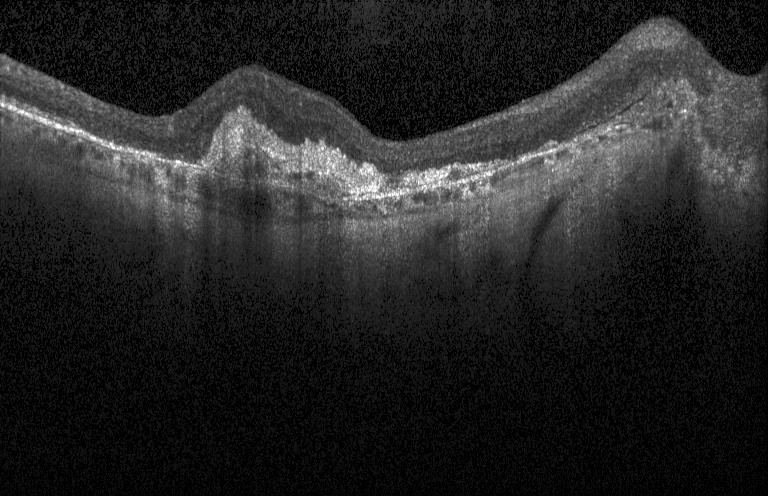 SD-OCT · OCT line scan — Diagnosis: CNV.